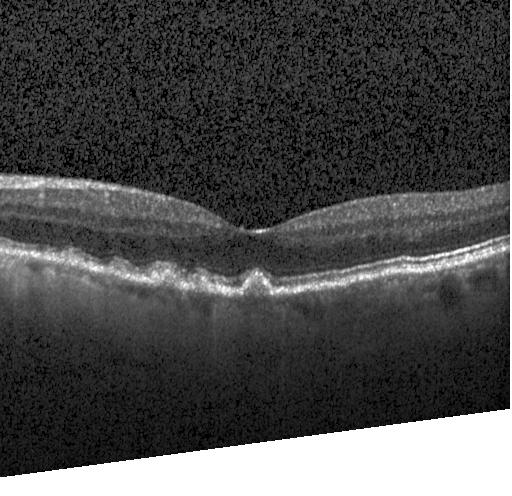
Spectral-domain optical coherence tomography · OCT B-scan · acquired on a Heidelberg Spectralis
Finding: sub-RPE drusenoid deposits.